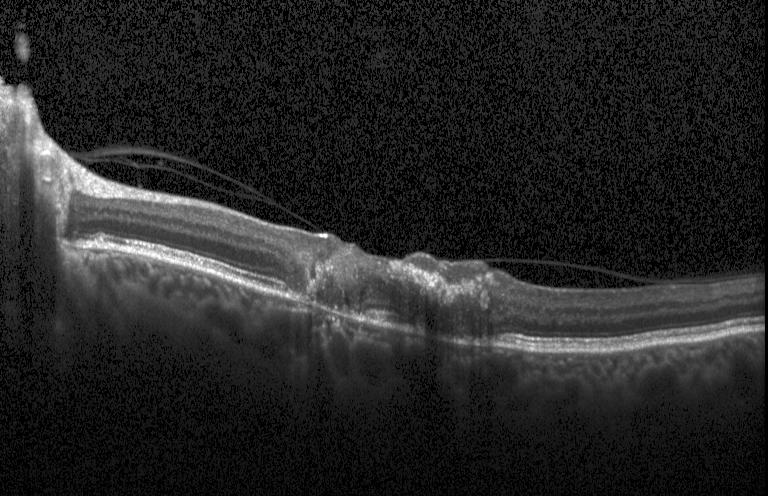 This B-scan demonstrates choroidal neovascularization.